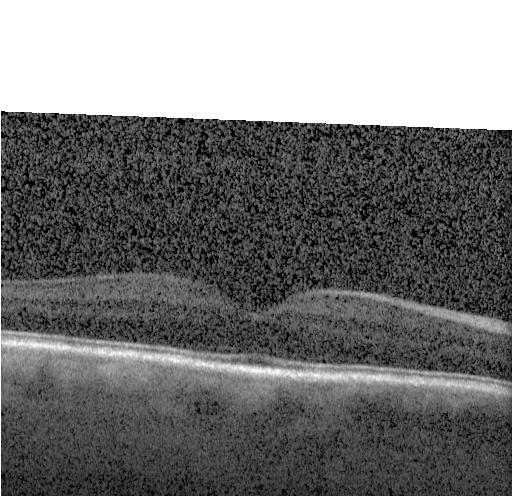
Retinal OCT cross-section
Impression: no CNV, DME, or drusen.